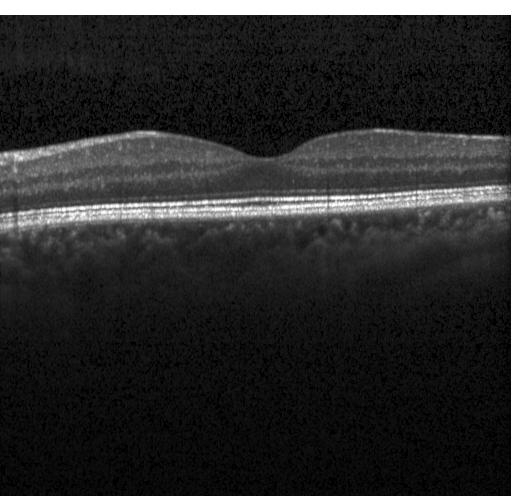
Diagnosis: no choroidal neovascularization, no diabetic macular edema, and no drusen.